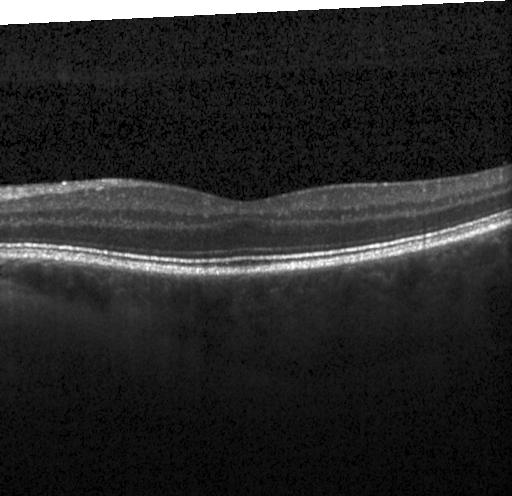

OCT scan showing no choroidal neovascularization, no diabetic macular edema, and no drusen.